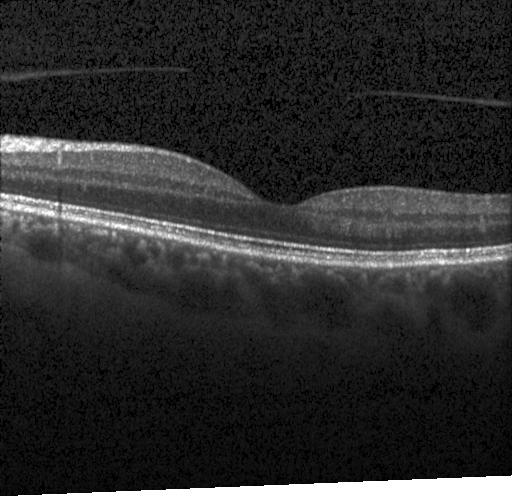
Retinal OCT B-scan. Macular OCT: no evidence of CNV, DME, or drusen.